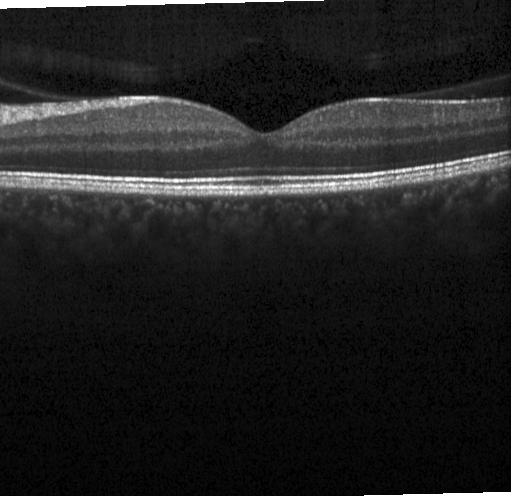

Heidelberg Spectralis · spectral-domain OCT · retinal OCT cross-section — Assessment: no choroidal neovascularization, no diabetic macular edema, and no drusen.